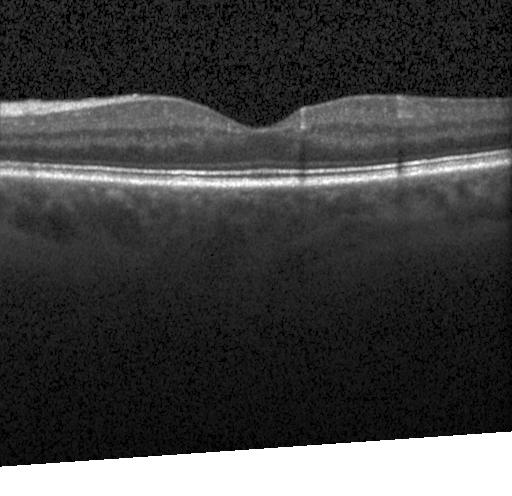 Diagnosis: neither CNV, DME, nor drusen.